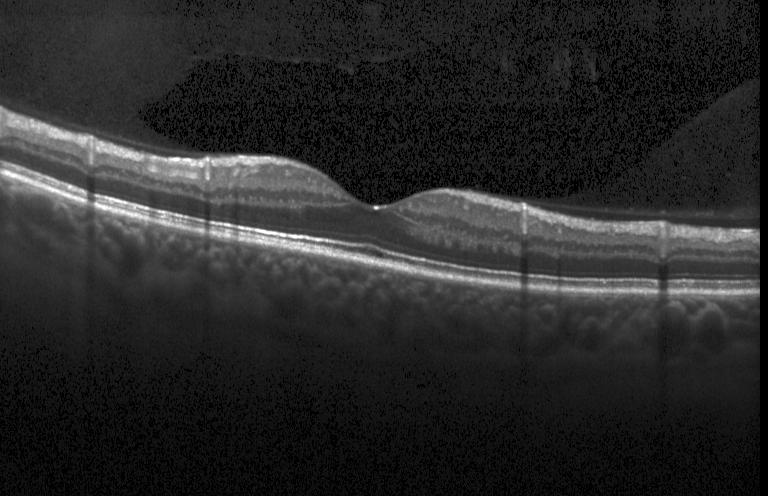

Diagnosis: no CNV, no DME, and no drusen.